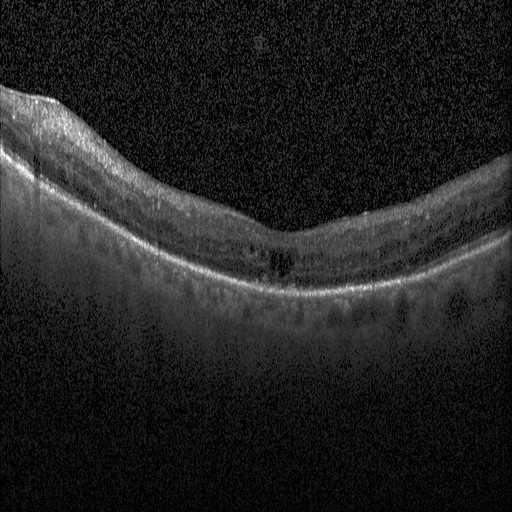

Instrument: Heidelberg Spectralis. OCT line scan. Spectral-domain OCT. Assessment: diabetic macular edema.